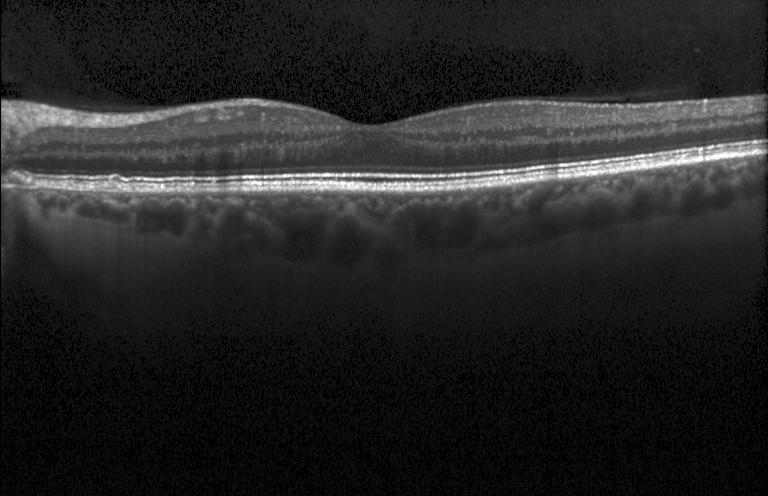 Impression: no evidence of CNV, DME, or drusen.